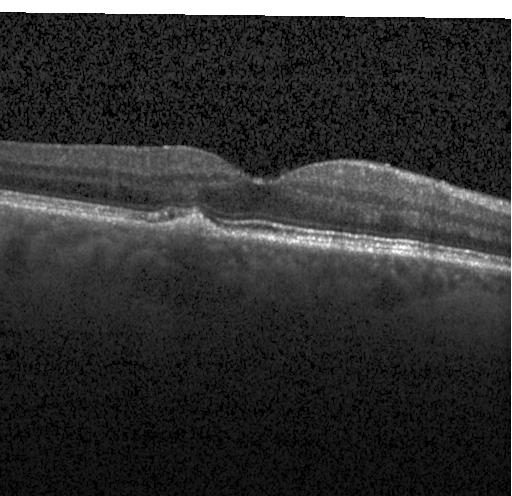
OCT B-scan showing sub-RPE drusenoid deposits.